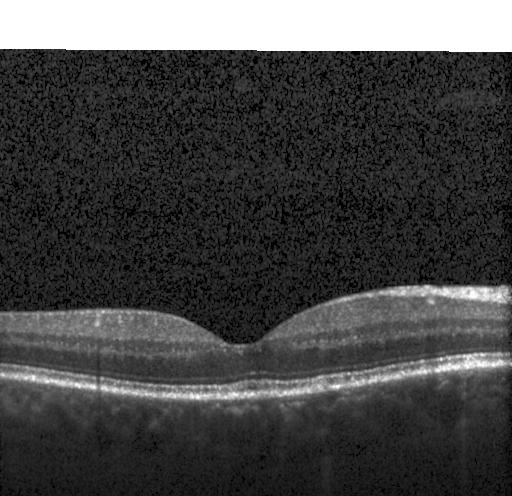 Acquired on a Heidelberg Spectralis, retinal OCT B-scan, spectral-domain optical coherence tomography.
Diagnosis: no choroidal neovascularization, diabetic macular edema, or drusen.